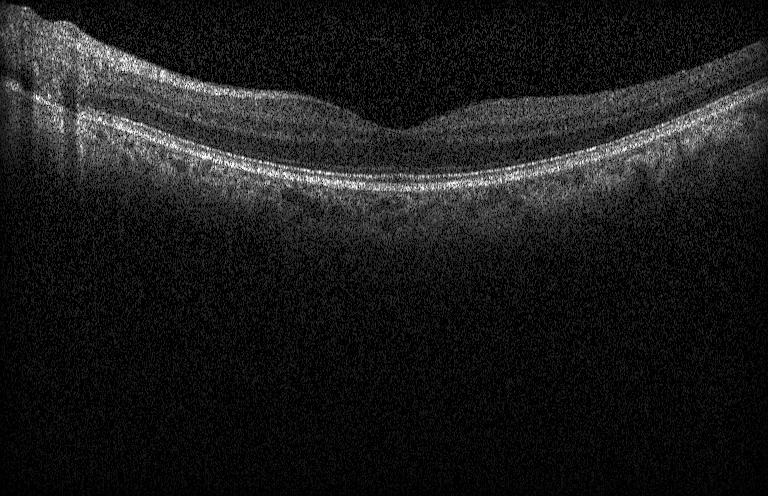
Finding: no choroidal neovascularization, no diabetic macular edema, and no drusen.